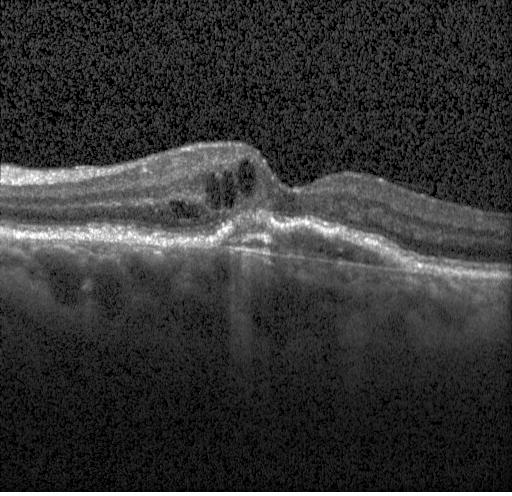

Retinal OCT cross-section, macular scan.
Finding: a choroidal neovascular membrane.